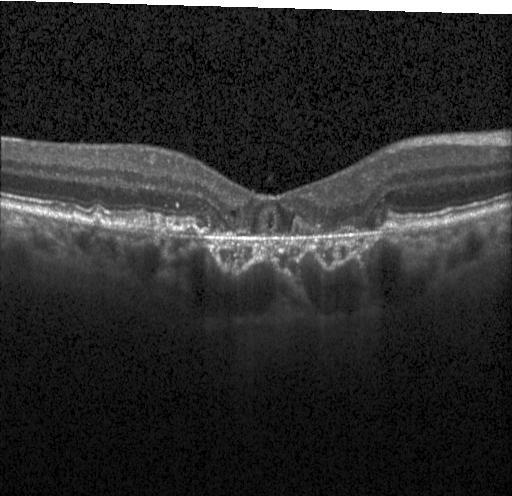
Optical coherence tomography B-scan · macular scan · spectral-domain OCT. Finding: choroidal neovascularization (CNV).